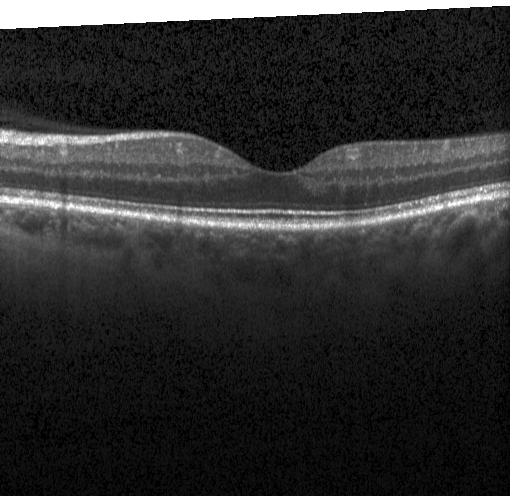

OCT B-scan — No CNV, no DME, and no drusen.